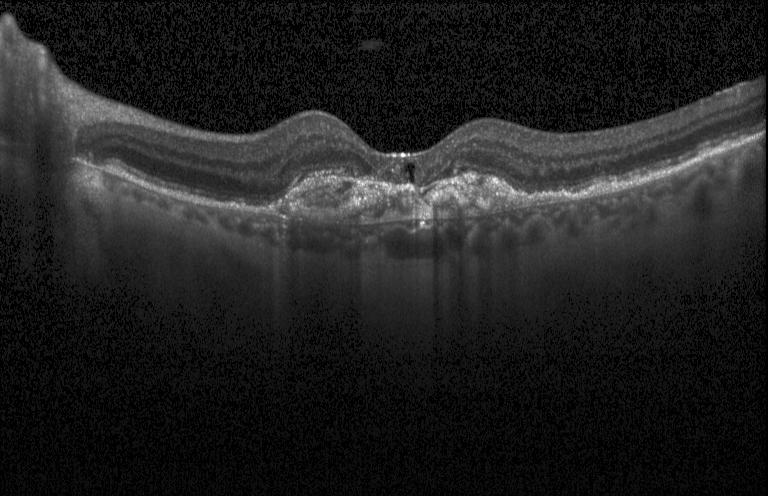 Finding: a choroidal neovascular membrane.